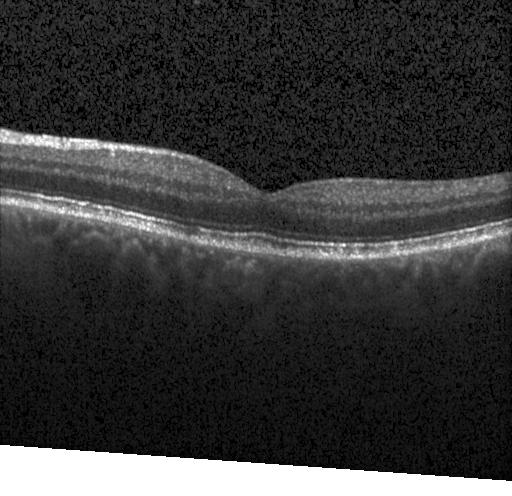 Spectral-domain OCT, OCT B-scan, through the macula. Diagnosis: no choroidal neovascularization, no diabetic macular edema, and no drusen.